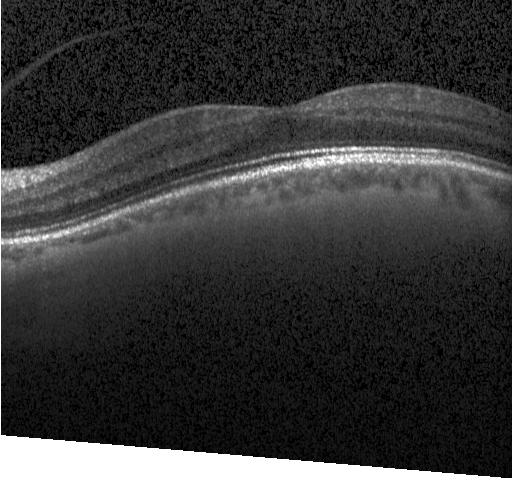
Centered on the fovea. OCT B-scan. Heidelberg Spectralis. SD-OCT
Macular OCT: no evidence of CNV, DME, or drusen.